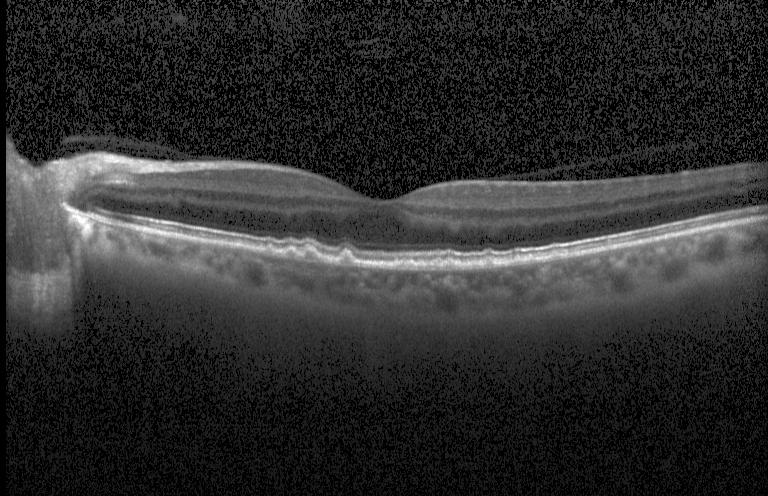

Impression: sub-RPE drusenoid deposits.